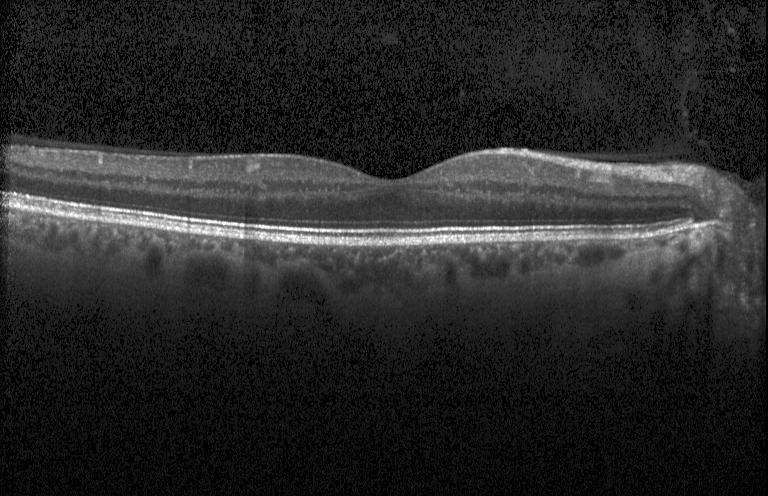 Retinal OCT B-scan.
Impression: no evidence of CNV, DME, or drusen.